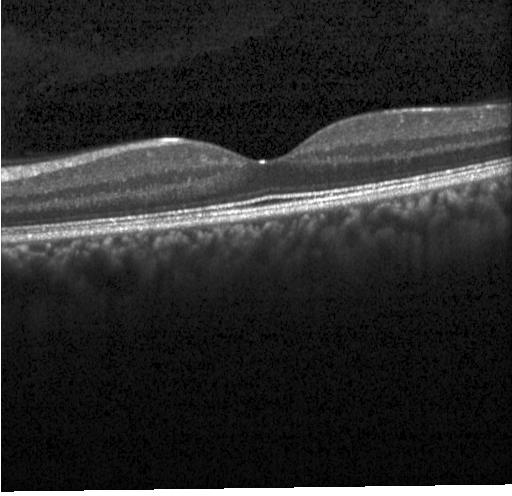

Acquired on a Heidelberg Spectralis, fovea-centered, OCT B-scan
This B-scan demonstrates no CNV, no DME, and no drusen.